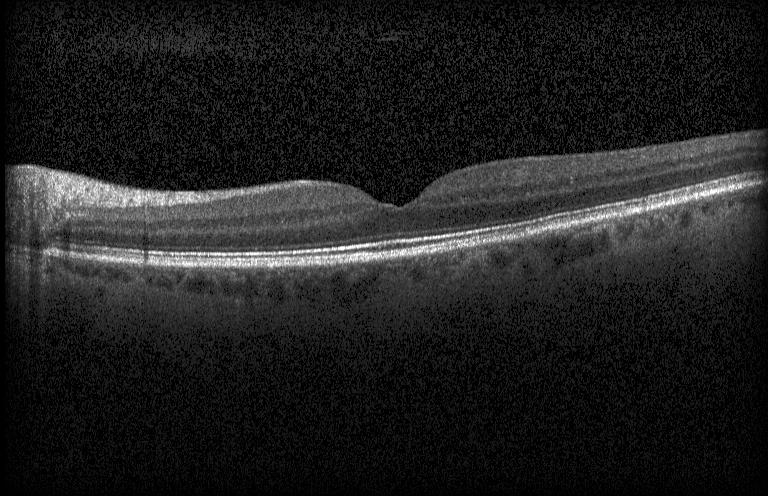 OCT B-scan showing no evidence of CNV, DME, or drusen.